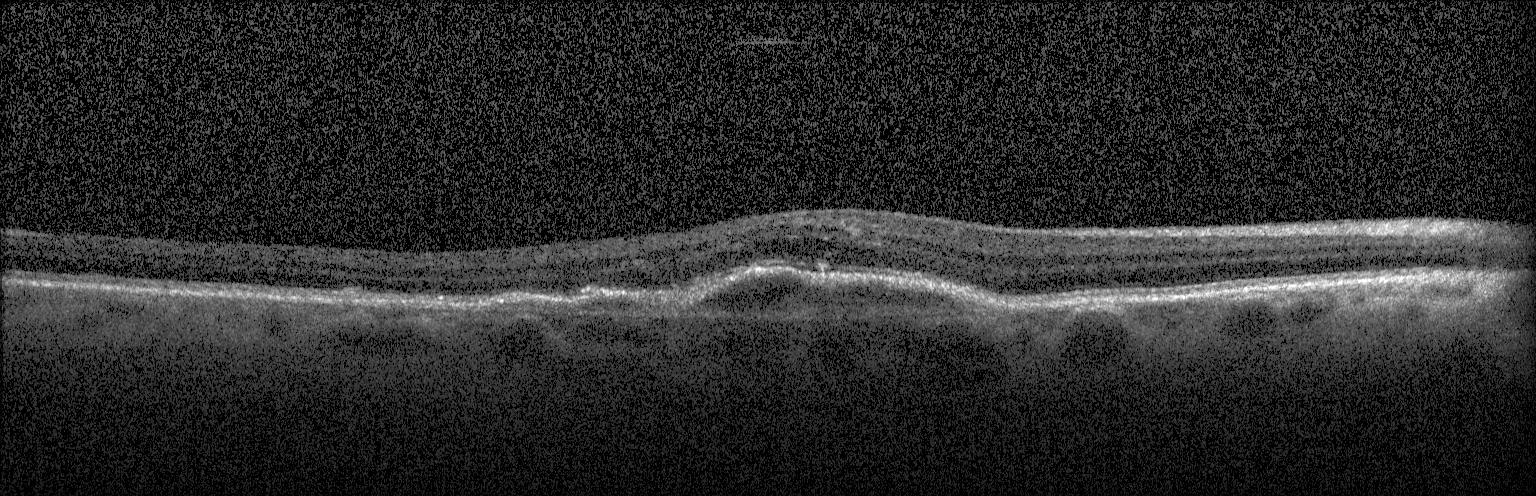
SD-OCT, OCT B-scan. Diagnosis: choroidal neovascularization.